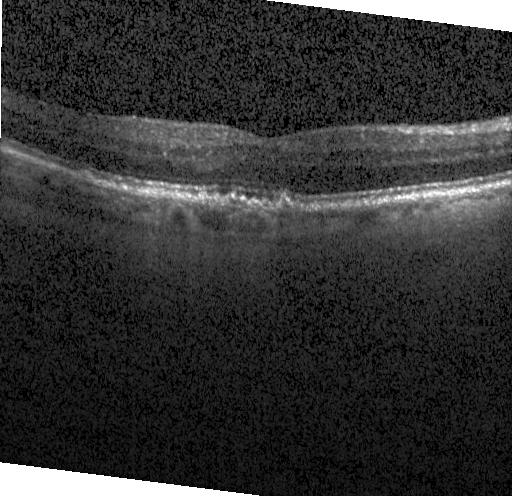 OCT B-scan · centered on the fovea · spectral-domain optical coherence tomography · Heidelberg Spectralis.
Sub-RPE drusenoid deposits.